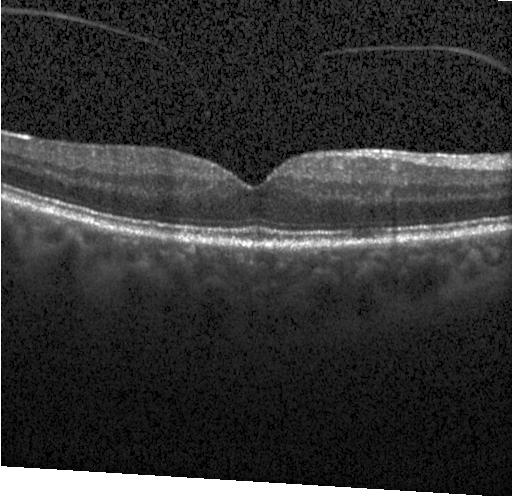

Spectral-domain OCT B-scan: no choroidal neovascularization, diabetic macular edema, or drusen.